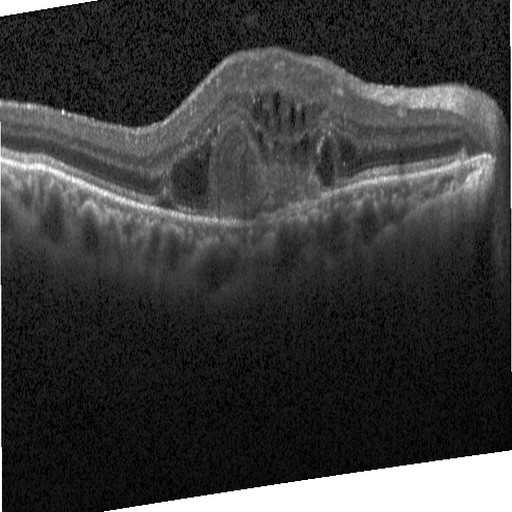 Diagnosis: diabetic macular edema.